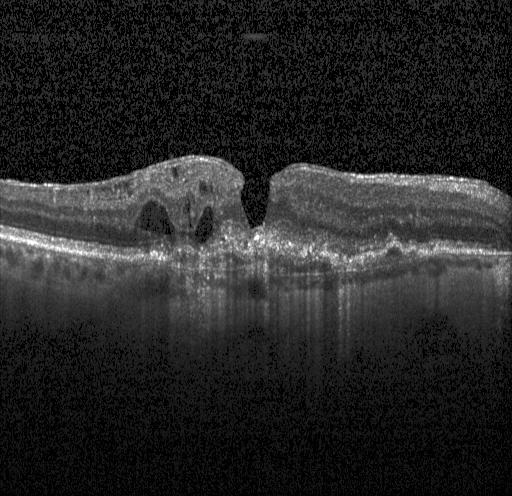

OCT scan showing a choroidal neovascular membrane.